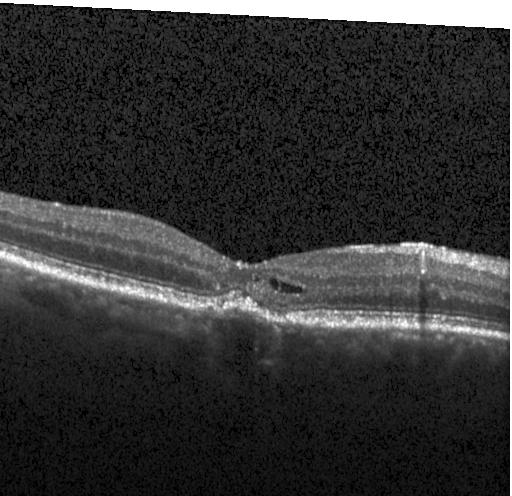

This B-scan demonstrates choroidal neovascularization.